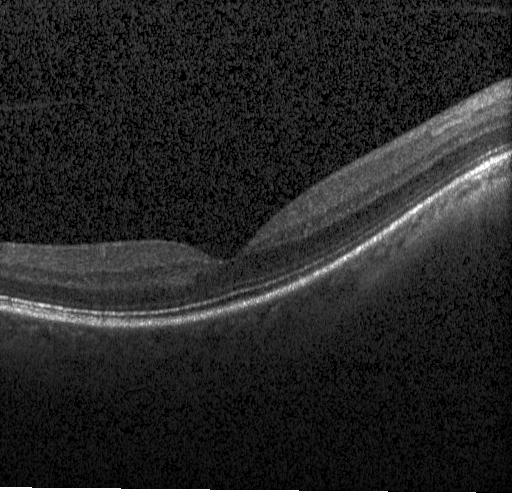 Optical coherence tomography scan. Finding: neither choroidal neovascularization, diabetic macular edema, nor drusen.